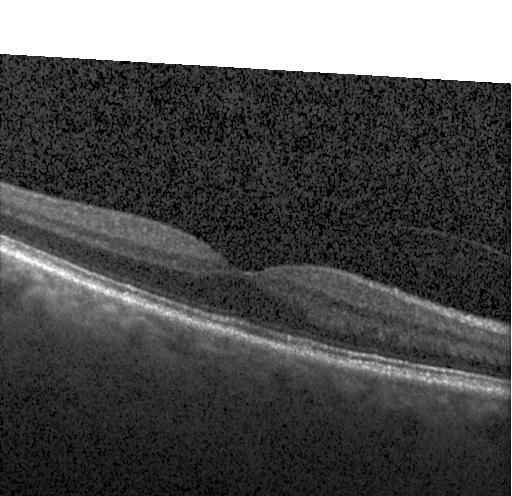

Optical coherence tomography B-scan, acquired on a Heidelberg Spectralis.
Diagnosis: no evidence of choroidal neovascularization, diabetic macular edema, or drusen.